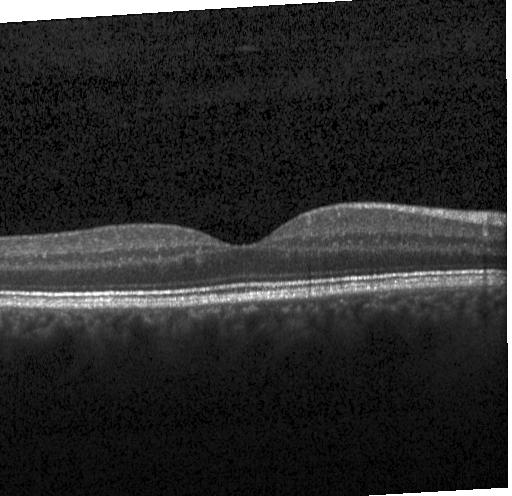
Retinal OCT cross-section showing neither CNV, DME, nor drusen.